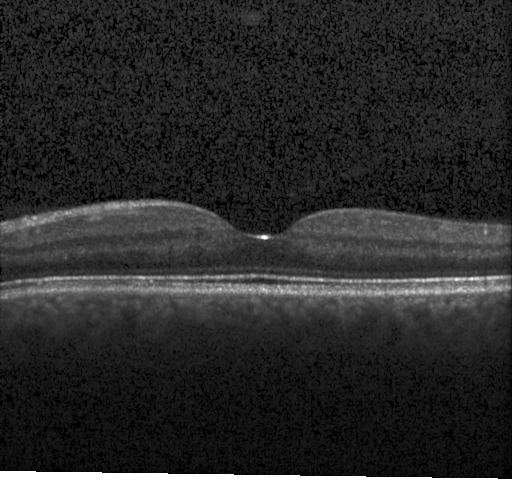 Impression: no evidence of choroidal neovascularization, diabetic macular edema, or drusen.